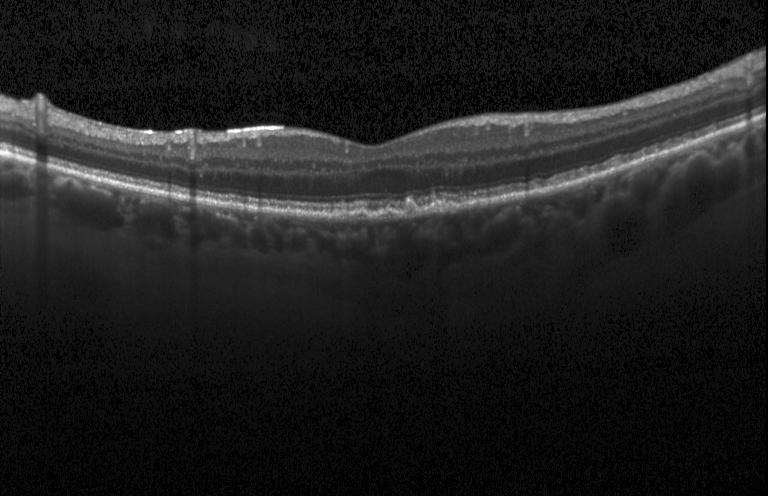 Macular OCT demonstrating drusen.